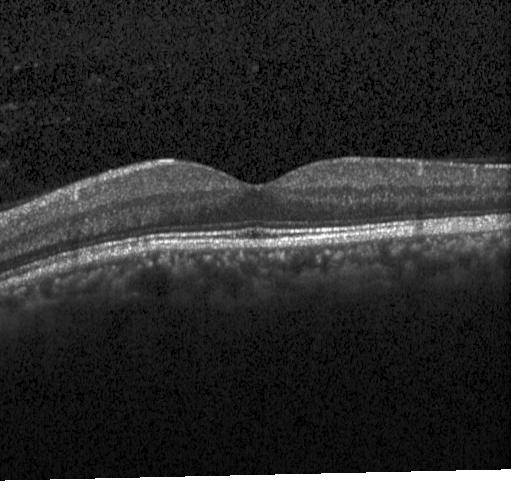
OCT line scan · spectral-domain optical coherence tomography · fovea-centered · instrument: Heidelberg Spectralis — Assessment: no CNV, no DME, and no drusen.